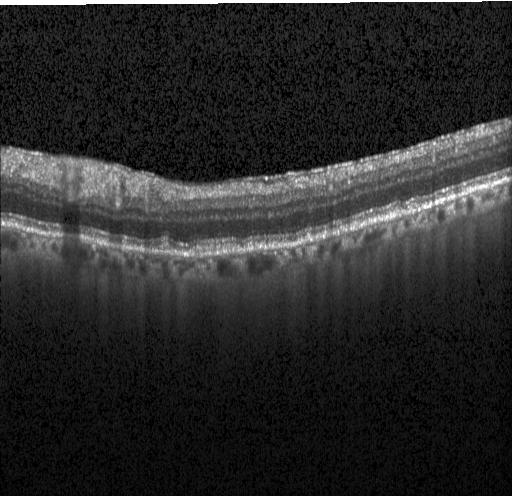 Horizontal scan through the fovea. Retinal OCT B-scan. Spectral-domain optical coherence tomography
Dx: sub-RPE drusenoid deposits.